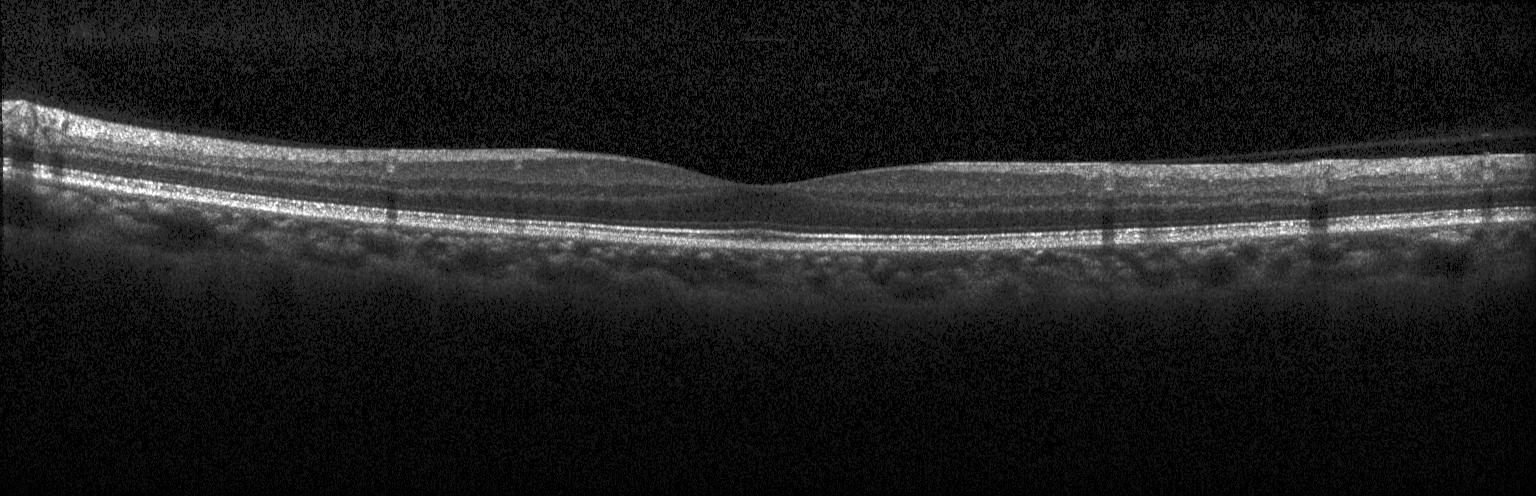

OCT finding: neither choroidal neovascularization, diabetic macular edema, nor drusen.